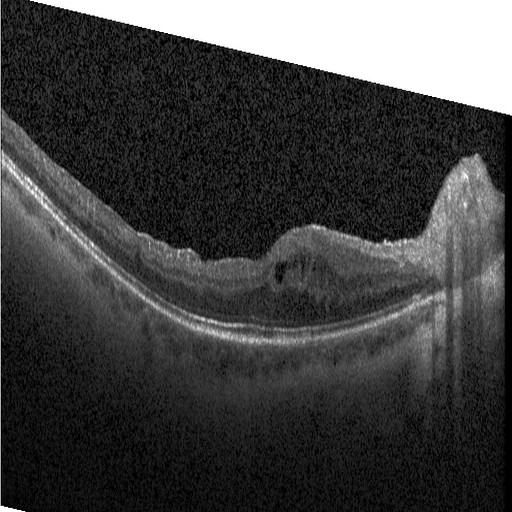

Centered on the fovea. Spectral-domain OCT. Optical coherence tomography B-scan — Impression: diabetic macular edema.